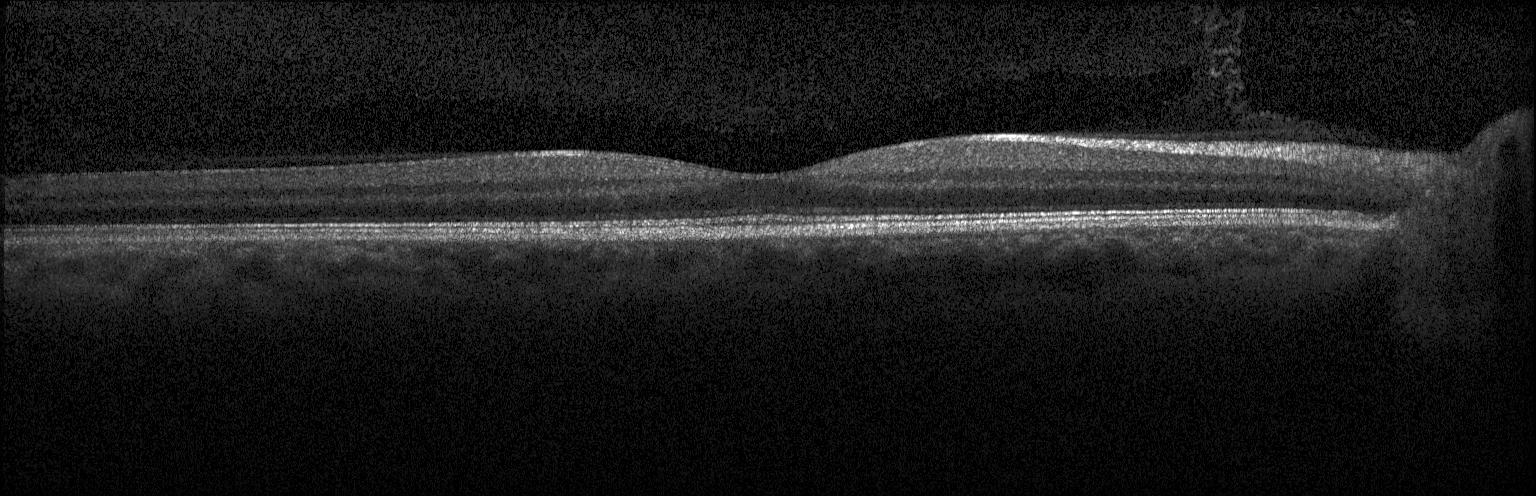
Retinal OCT B-scan.
OCT finding: no evidence of choroidal neovascularization, diabetic macular edema, or drusen.